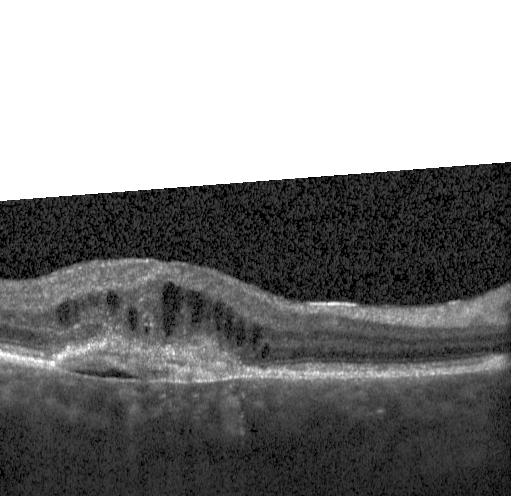 Macular scan, retinal OCT cross-section, spectral-domain OCT. OCT finding: CNV.